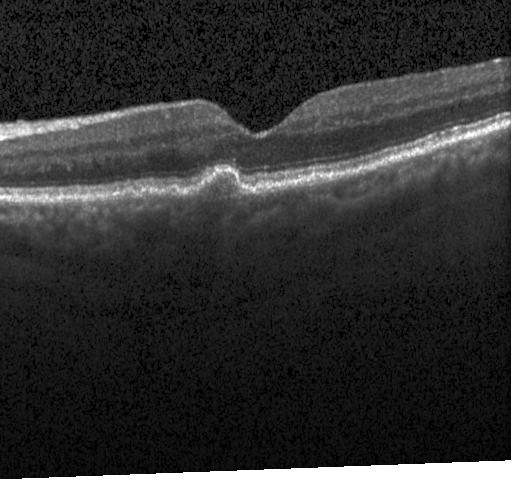
Impression: multiple drusen.